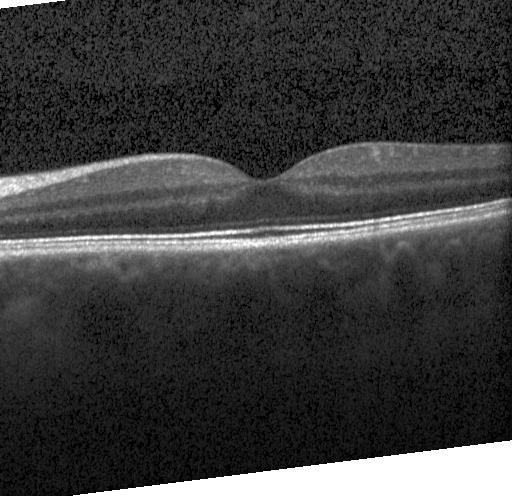

No choroidal neovascularization, no diabetic macular edema, and no drusen.